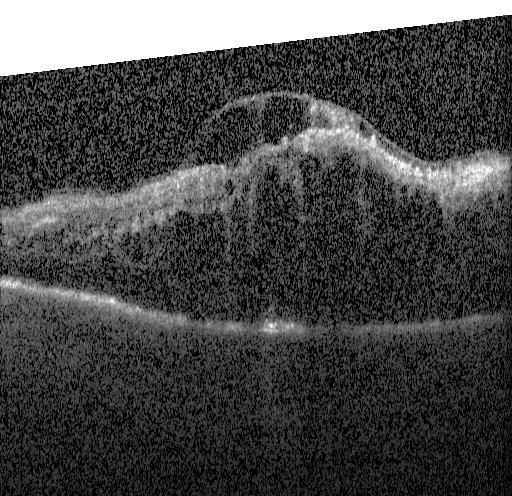 Finding: DME.